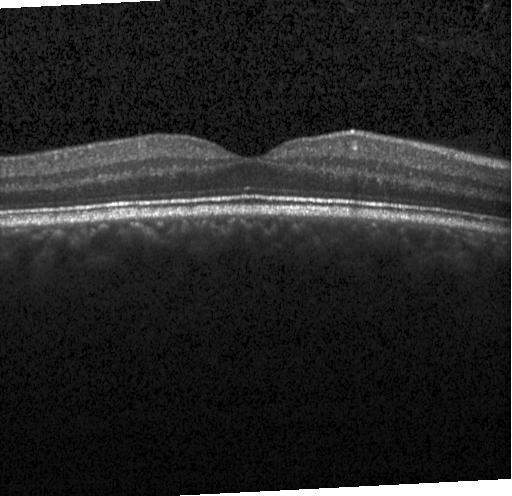
OCT line scan; centered on the fovea. This B-scan demonstrates no CNV, DME, or drusen.